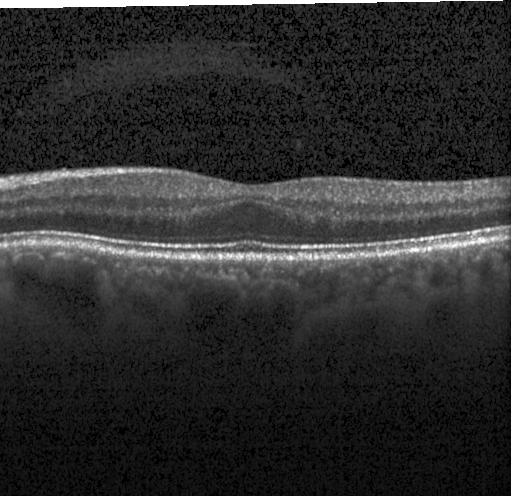

Heidelberg Spectralis; retinal OCT B-scan
Diagnosis: no evidence of choroidal neovascularization, diabetic macular edema, or drusen.